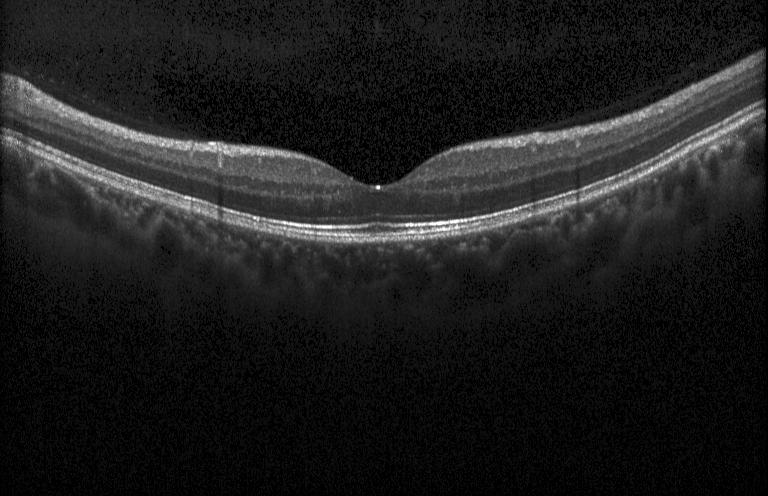 Heidelberg Spectralis. SD-OCT. Through the macula. OCT B-scan. The scan shows neither CNV, DME, nor drusen.